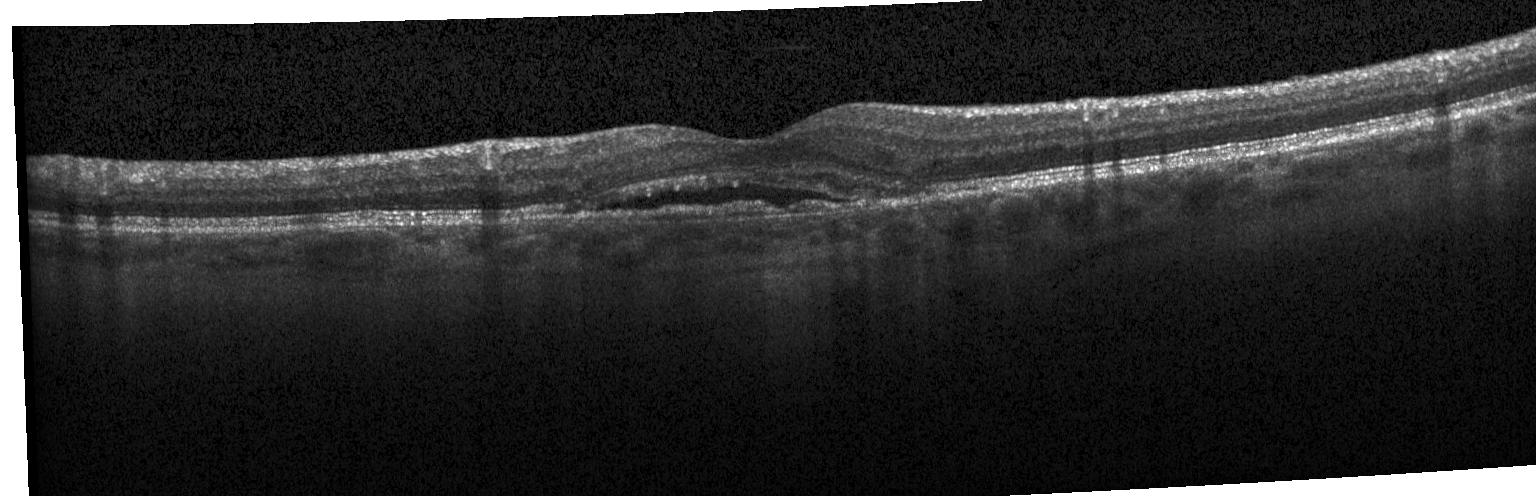

Retinal OCT B-scan
Impression: CNV.